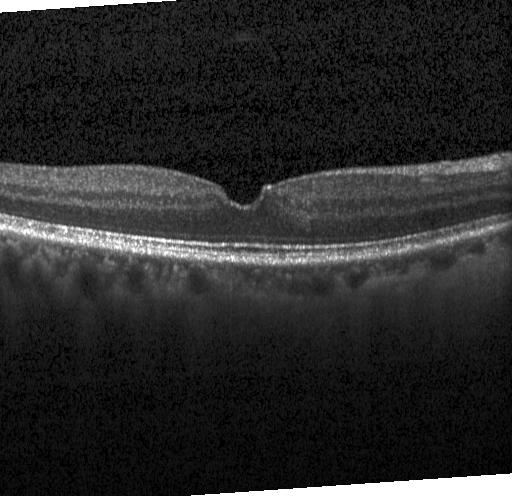

Retinal OCT B-scan · fovea-centered · instrument: Heidelberg Spectralis
Diagnosis: no choroidal neovascularization, diabetic macular edema, or drusen.